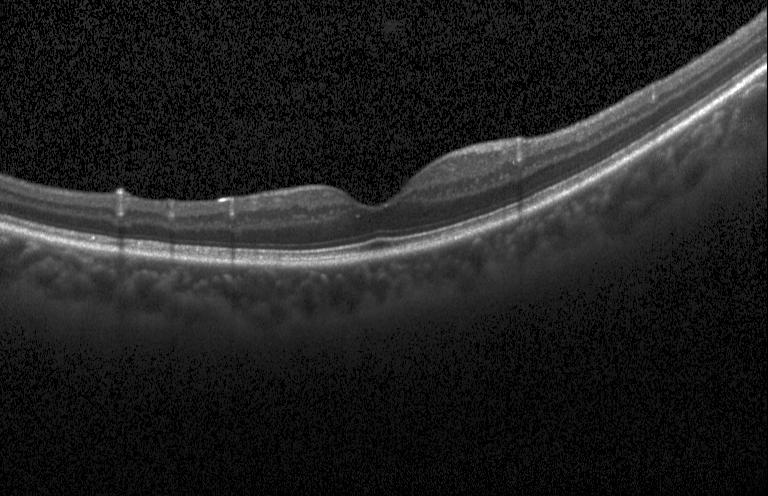
Finding: neither choroidal neovascularization, diabetic macular edema, nor drusen.